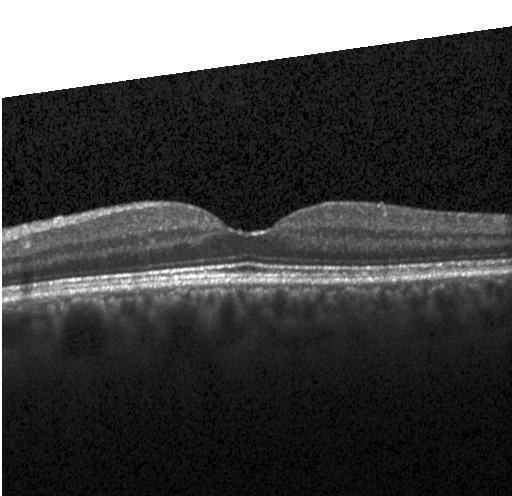

This B-scan demonstrates neither CNV, DME, nor drusen.